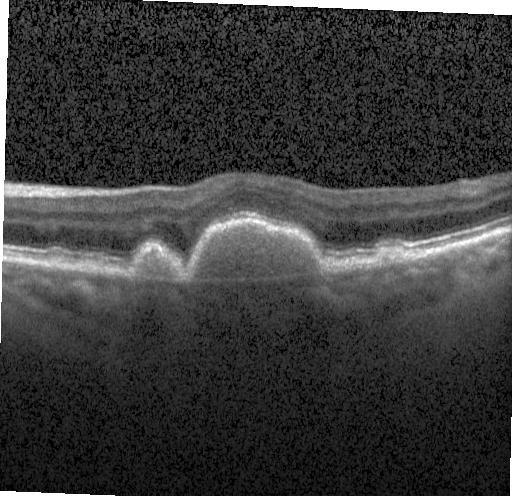

Finding: choroidal neovascularization.